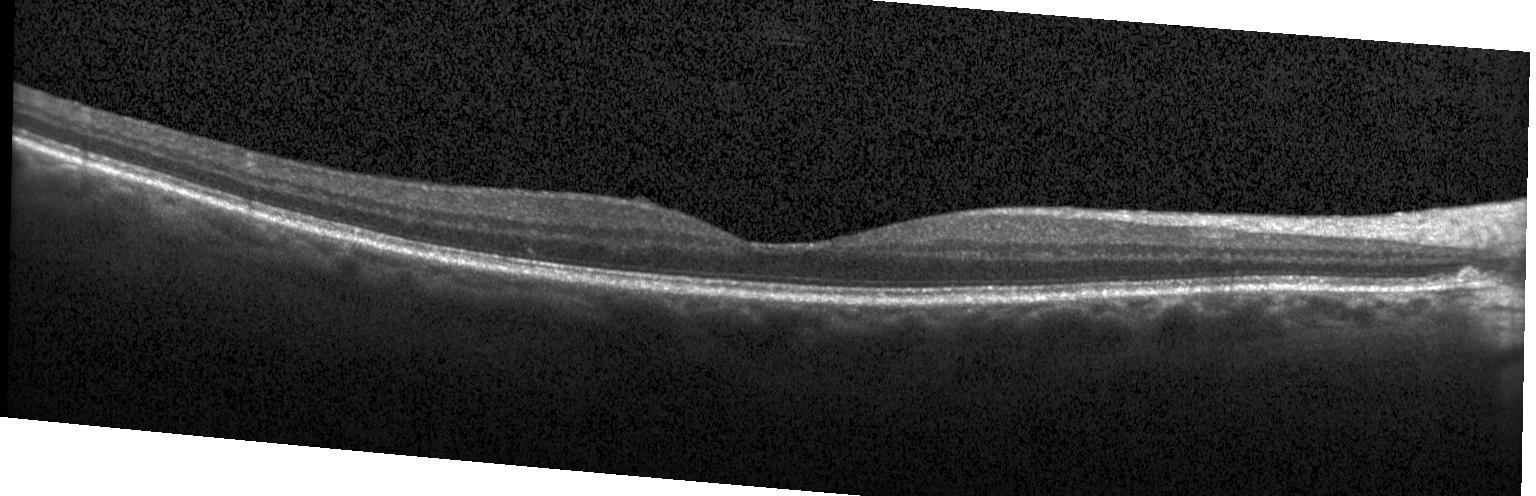

Macular OCT: no choroidal neovascularization, diabetic macular edema, or drusen.